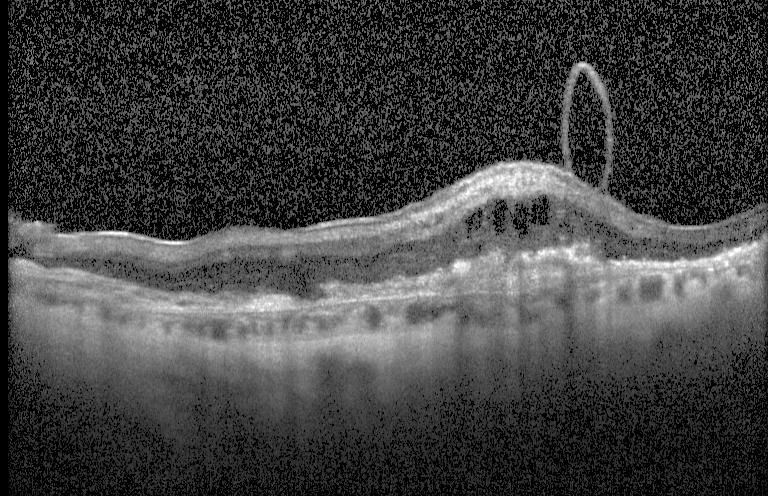
Spectral-domain optical coherence tomography. Heidelberg Spectralis. Retinal OCT B-scan. Diagnosis: choroidal neovascularization.